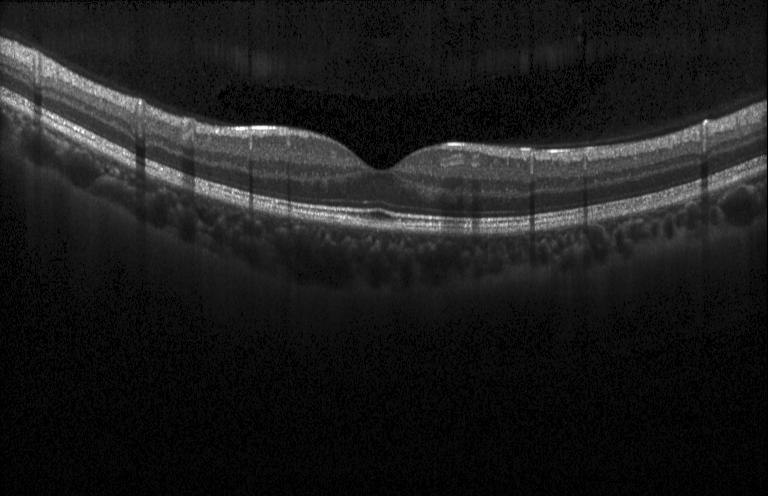
Impression: no CNV, DME, or drusen.